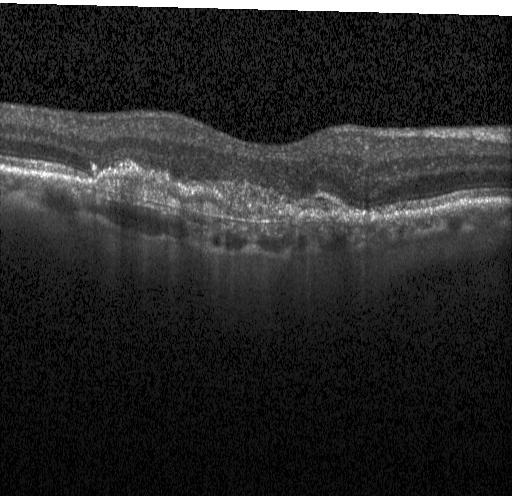
Fovea-centered · SD-OCT · acquired on a Heidelberg Spectralis · retinal OCT B-scan.
This B-scan demonstrates choroidal neovascularization (CNV).